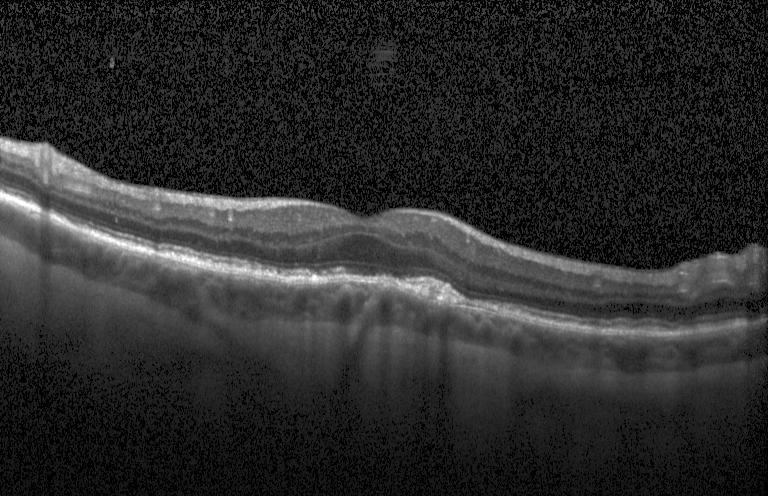 Finding: choroidal neovascularization.